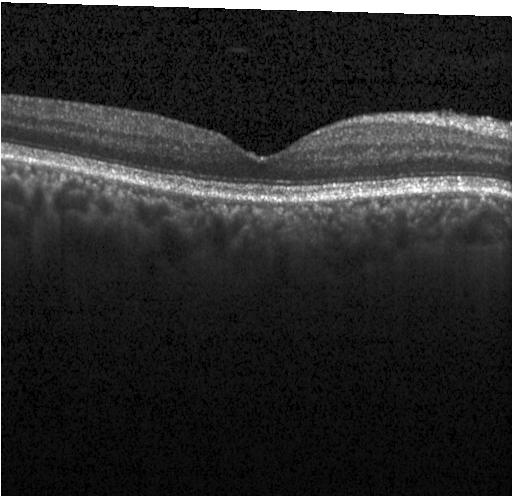 Heidelberg Spectralis OCT system · retinal OCT B-scan · spectral-domain optical coherence tomography · horizontal scan through the fovea
Finding: neither choroidal neovascularization, diabetic macular edema, nor drusen.